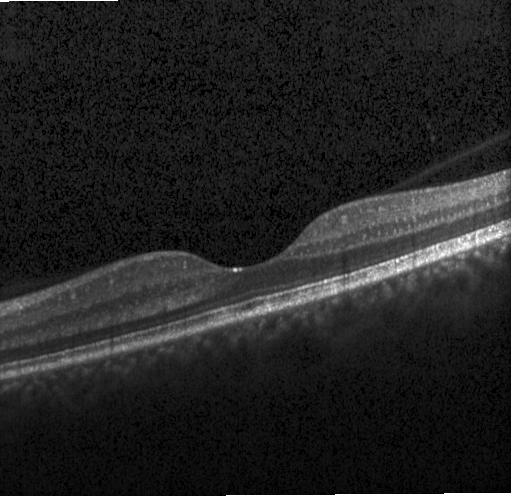

Optical coherence tomography B-scan.
The scan shows no choroidal neovascularization, diabetic macular edema, or drusen.